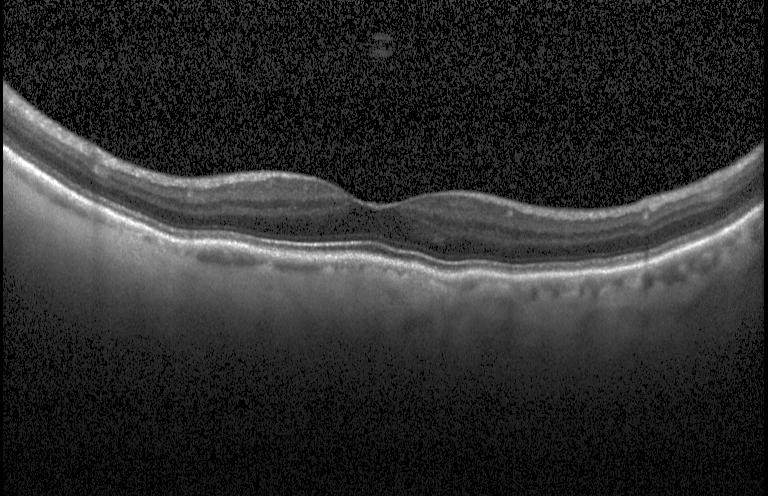 Dx: no CNV, no DME, and no drusen.